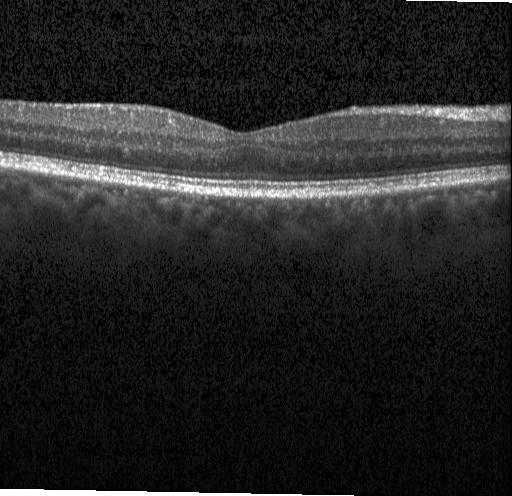

Heidelberg Spectralis; optical coherence tomography B-scan; spectral-domain OCT; centered on the fovea.
Diagnosis: no evidence of CNV, DME, or drusen.